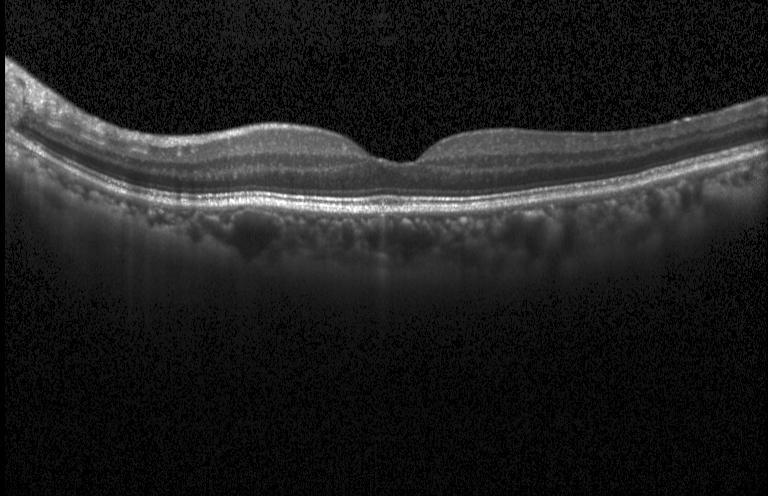

Fovea-centered, instrument: Heidelberg Spectralis, spectral-domain optical coherence tomography, retinal OCT cross-section — Finding: neither choroidal neovascularization, diabetic macular edema, nor drusen.